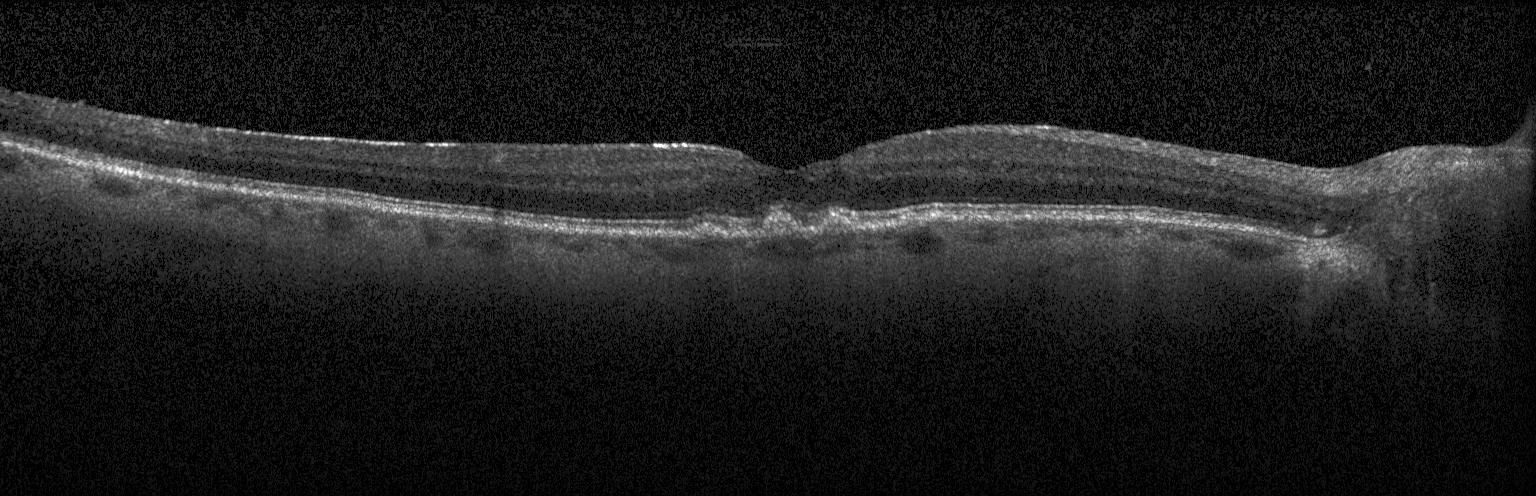 Diagnosis: drusen.